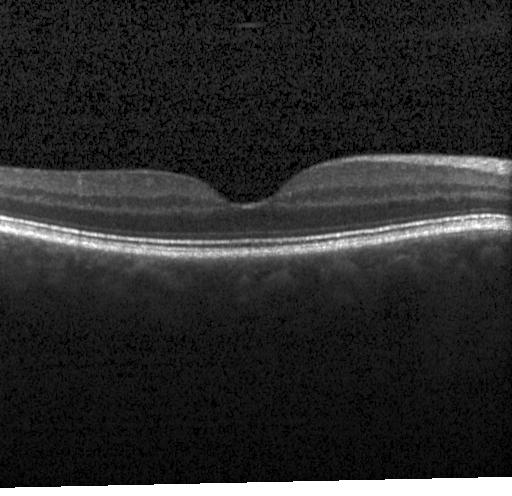
Heidelberg Spectralis, OCT B-scan, horizontal scan through the fovea, spectral-domain optical coherence tomography. The scan shows neither CNV, DME, nor drusen.